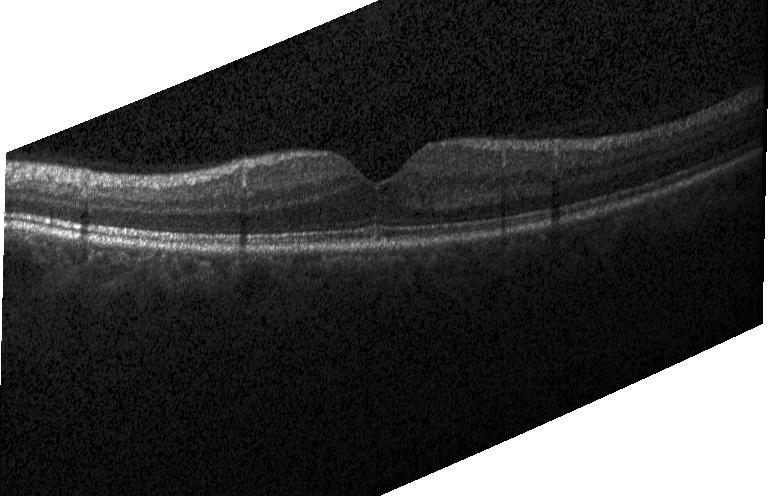

Optical coherence tomography B-scan
This B-scan demonstrates no choroidal neovascularization, no diabetic macular edema, and no drusen.